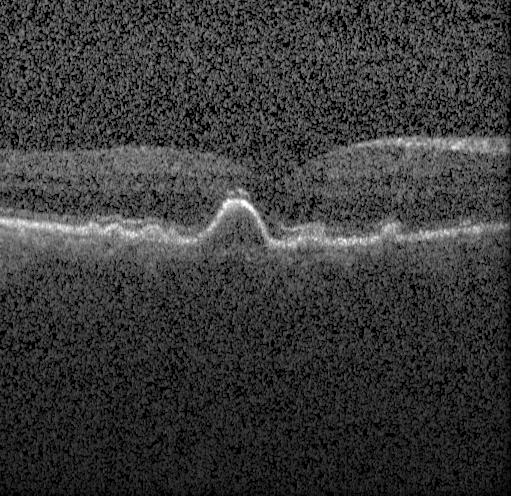 Diagnosis: multiple drusen.